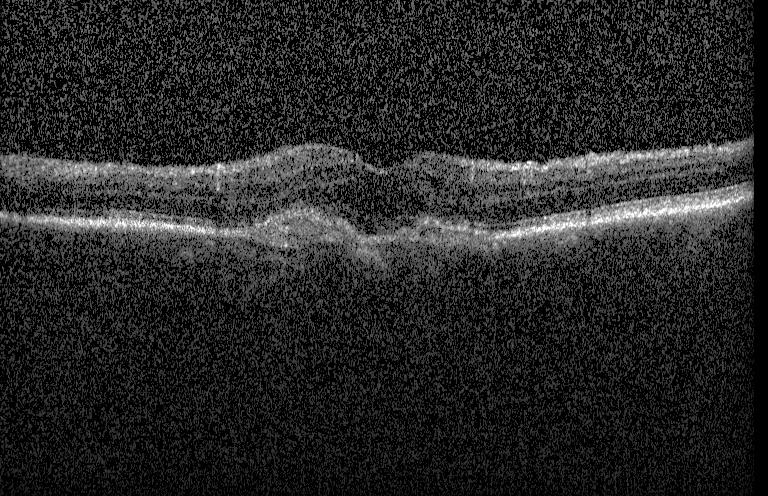 Diagnosis: a choroidal neovascular membrane.